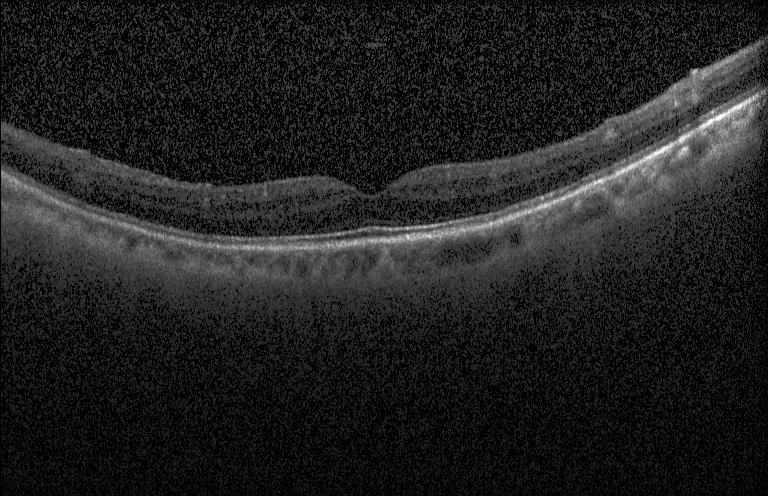
Optical coherence tomography scan · horizontal scan through the fovea · SD-OCT · Heidelberg Spectralis OCT system
Diagnosis: no choroidal neovascularization, no diabetic macular edema, and no drusen.